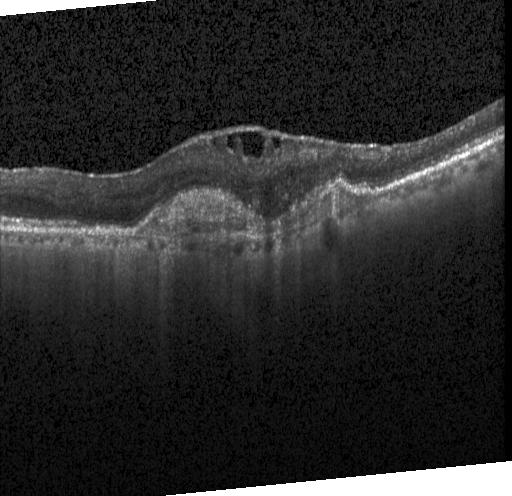 CNV.